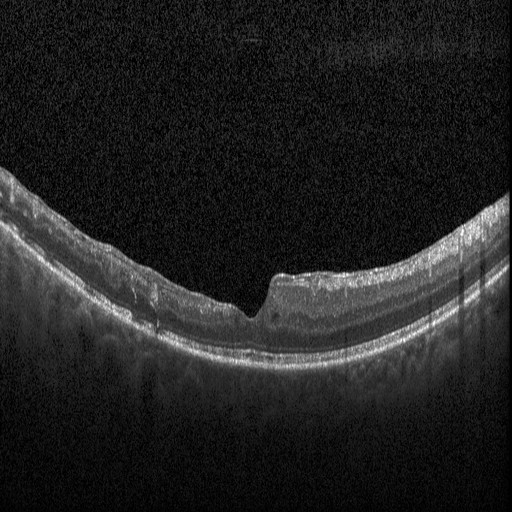
Instrument: Heidelberg Spectralis · retinal OCT cross-section · SD-OCT · horizontal scan through the fovea — Diagnosis: diabetic macular edema (DME).